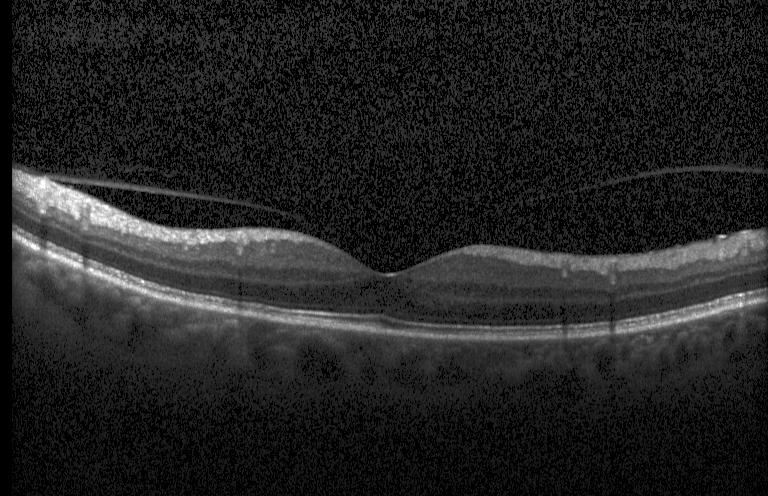
Finding: no choroidal neovascularization, no diabetic macular edema, and no drusen.